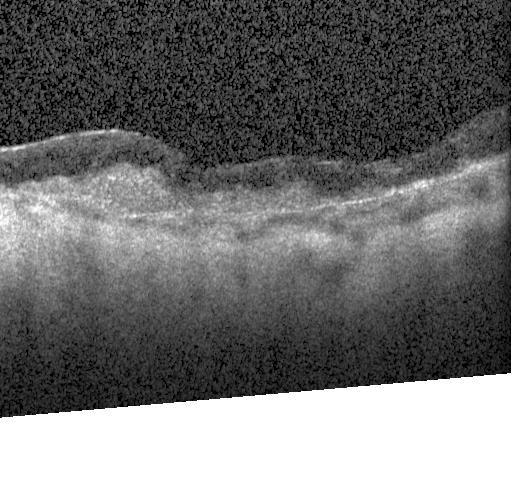
Retinal OCT cross-section showing a choroidal neovascular membrane.